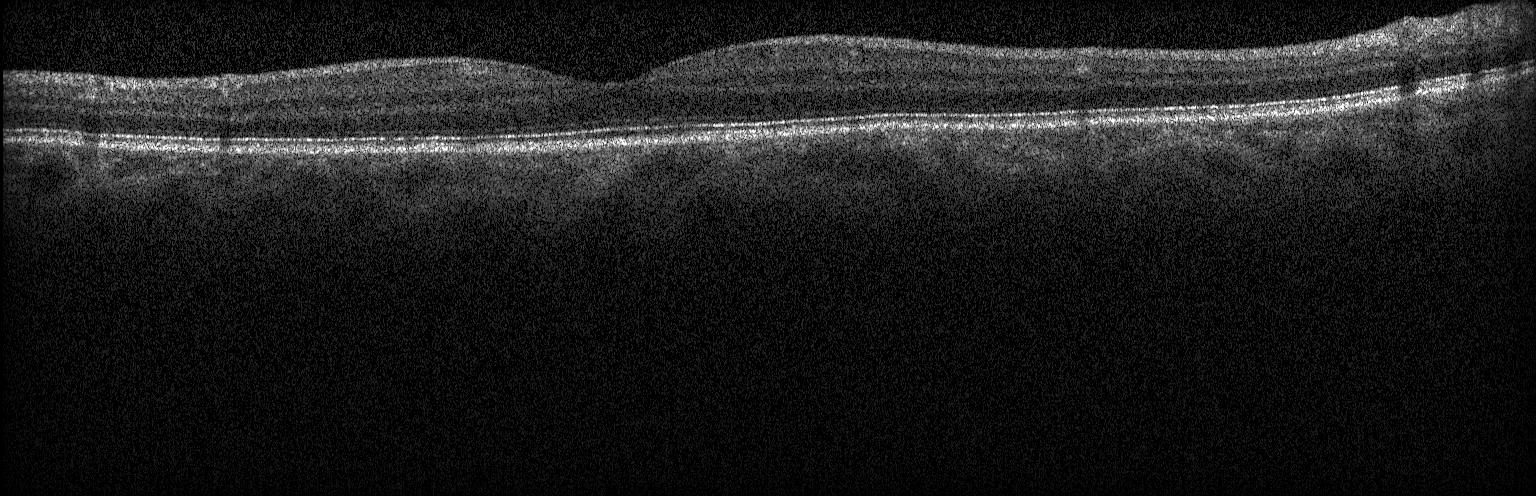 Macular OCT demonstrating no choroidal neovascularization, diabetic macular edema, or drusen.